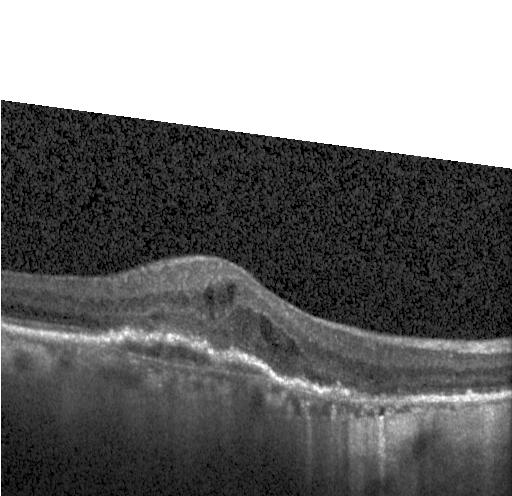
Retinal OCT B-scan.
The scan shows choroidal neovascularization.